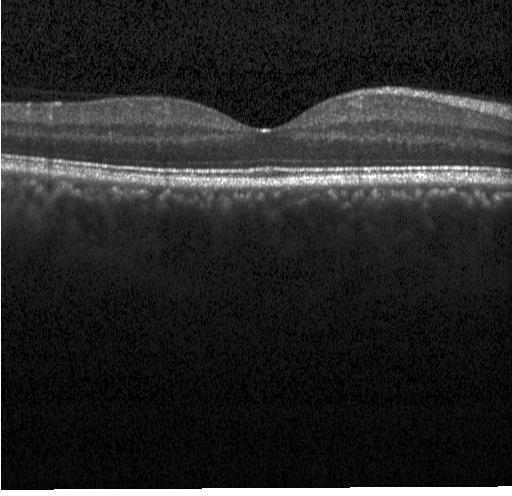 Spectral-domain optical coherence tomography, retinal OCT cross-section, macular scan. Assessment: neither choroidal neovascularization, diabetic macular edema, nor drusen.